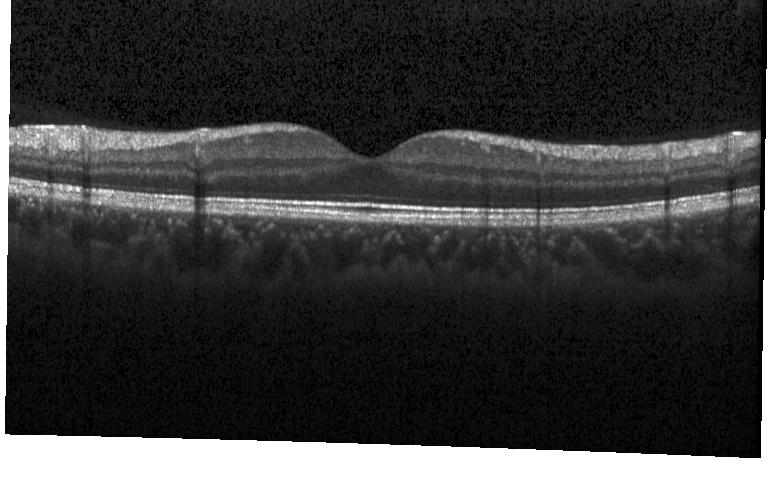 Retinal OCT cross-section.
Diagnosis: no evidence of CNV, DME, or drusen.